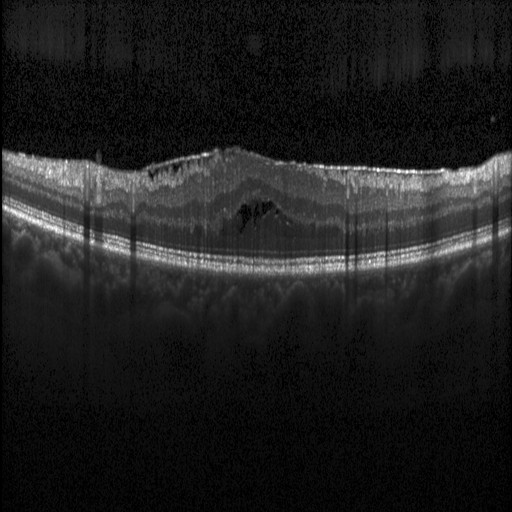 Spectral-domain optical coherence tomography. Acquired on a Heidelberg Spectralis. Retinal OCT B-scan. Finding: diabetic macular edema.